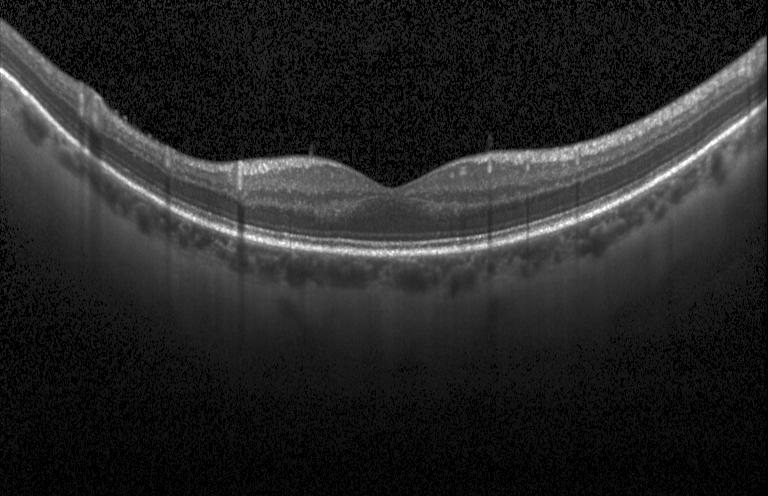

Retinal OCT B-scan
Neither choroidal neovascularization, diabetic macular edema, nor drusen.